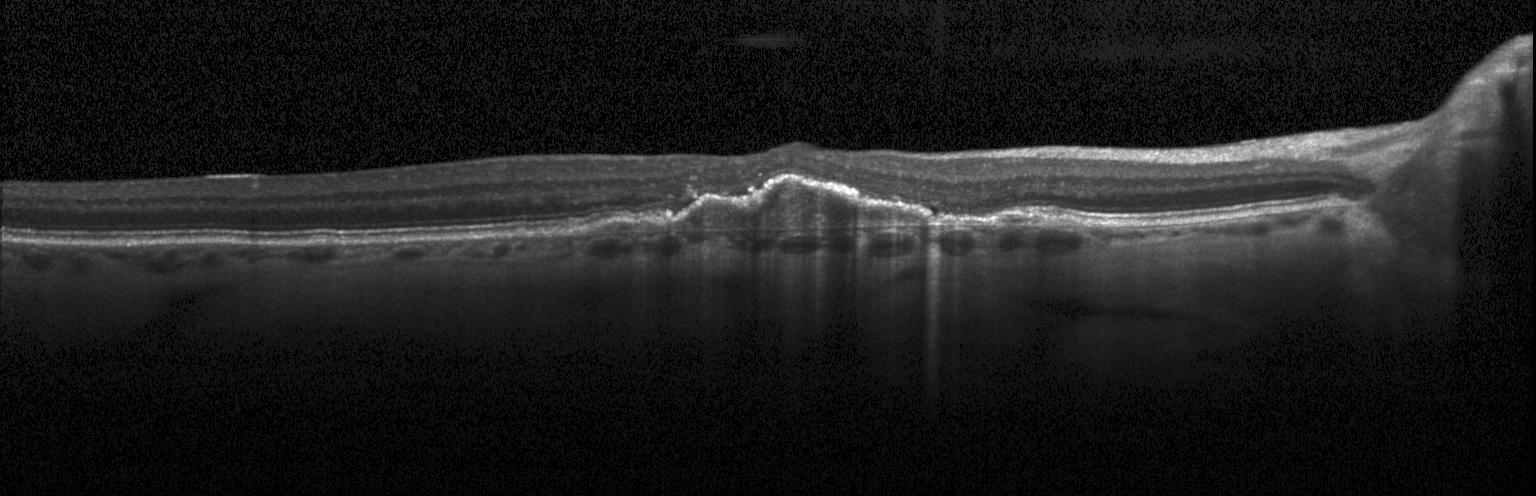

Retinal OCT B-scan.
Macular OCT: choroidal neovascularization.